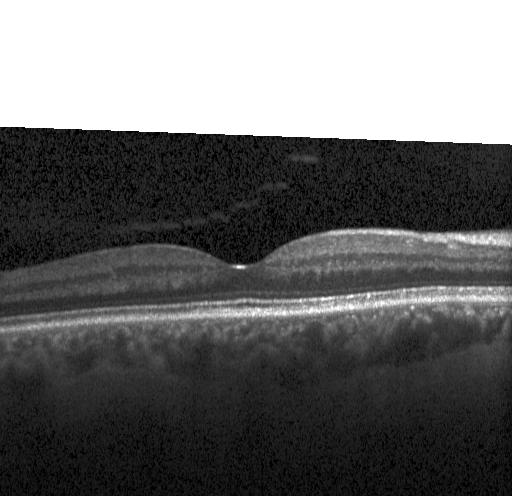 Spectral-domain OCT B-scan: no choroidal neovascularization, no diabetic macular edema, and no drusen.